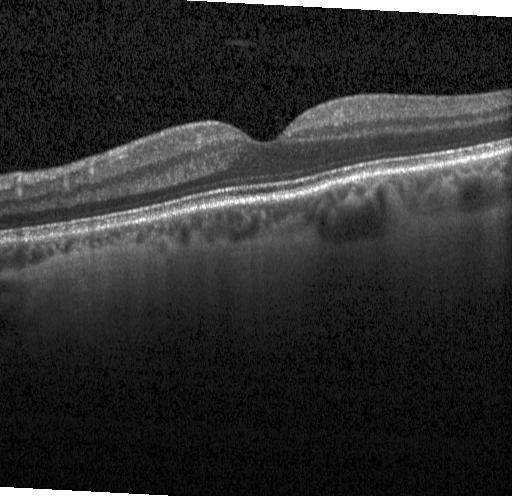 Retinal OCT B-scan · centered on the fovea.
Diagnosis: no CNV, DME, or drusen.